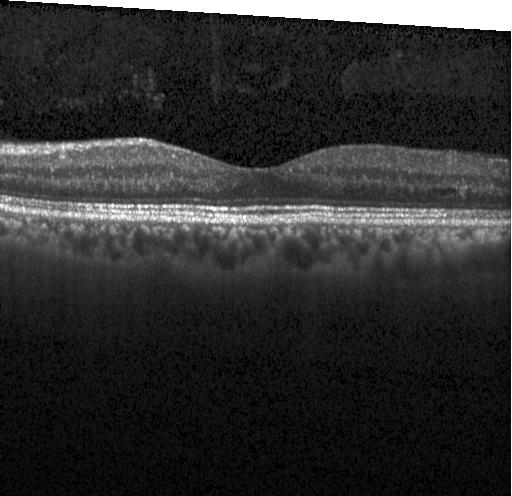
Optical coherence tomography B-scan, spectral-domain OCT. Finding: neither choroidal neovascularization, diabetic macular edema, nor drusen.